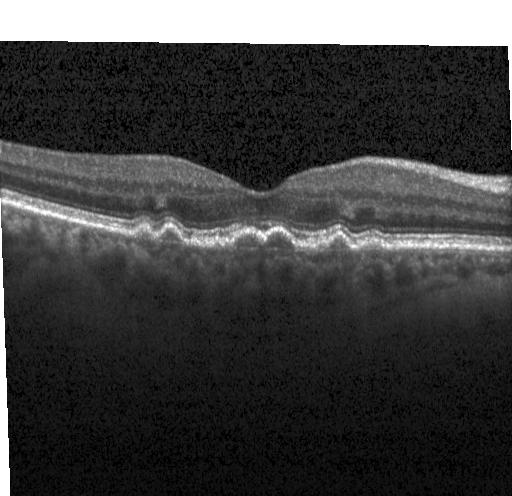 Acquired on a Heidelberg Spectralis; through the macula; optical coherence tomography B-scan; spectral-domain optical coherence tomography — Dx: sub-RPE drusenoid deposits.